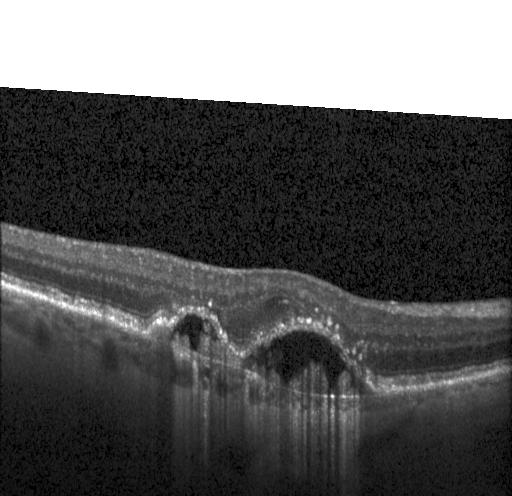 SD-OCT; horizontal scan through the fovea; OCT B-scan.
Dx: a choroidal neovascular membrane.